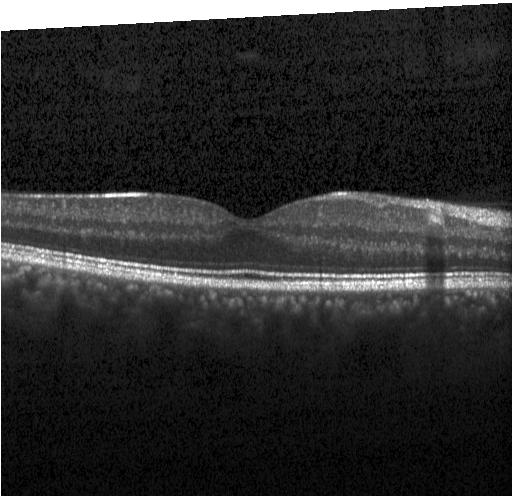

OCT line scan, Heidelberg Spectralis OCT system, SD-OCT, through the macula.
Impression: neither CNV, DME, nor drusen.